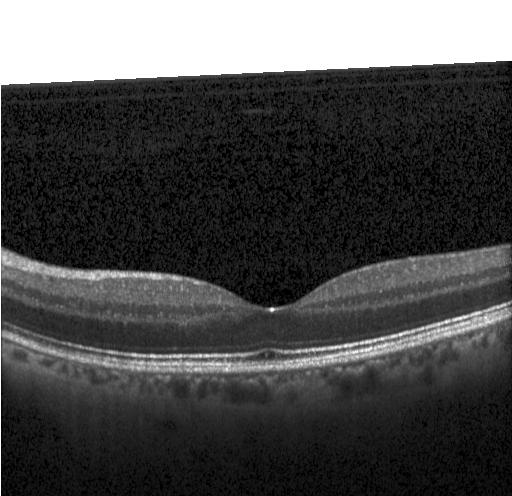 Retinal OCT cross-section — No CNV, DME, or drusen.